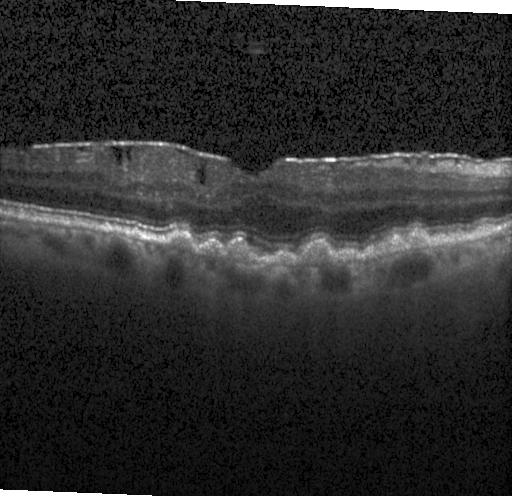 OCT B-scan showing multiple drusen.